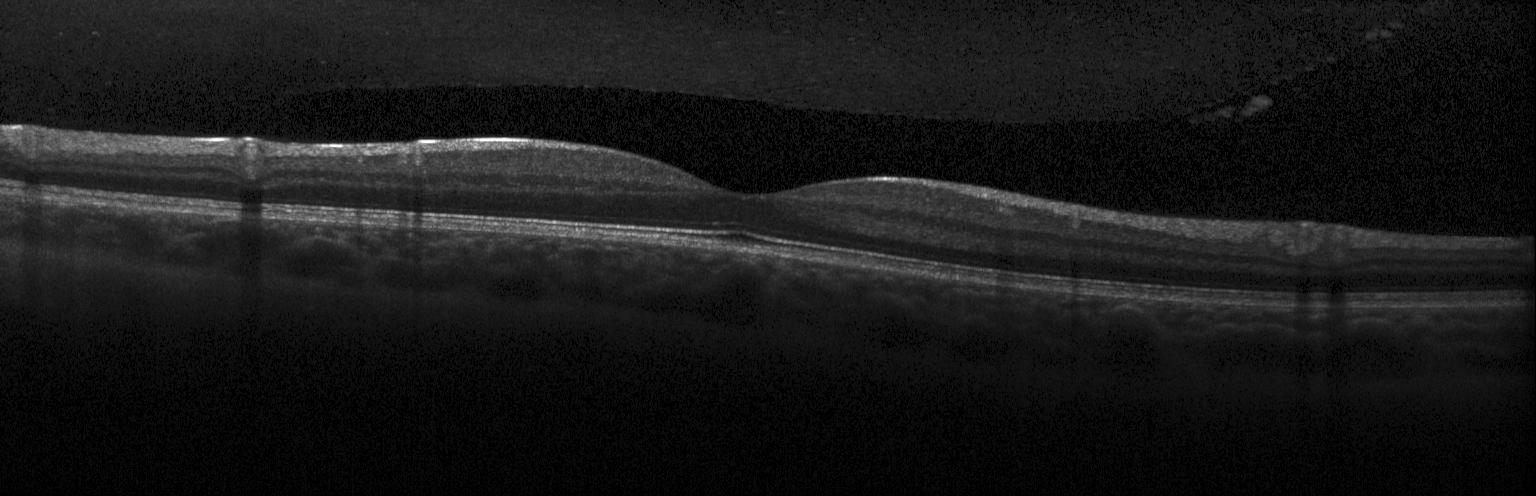

Optical coherence tomography B-scan. No CNV, DME, or drusen.